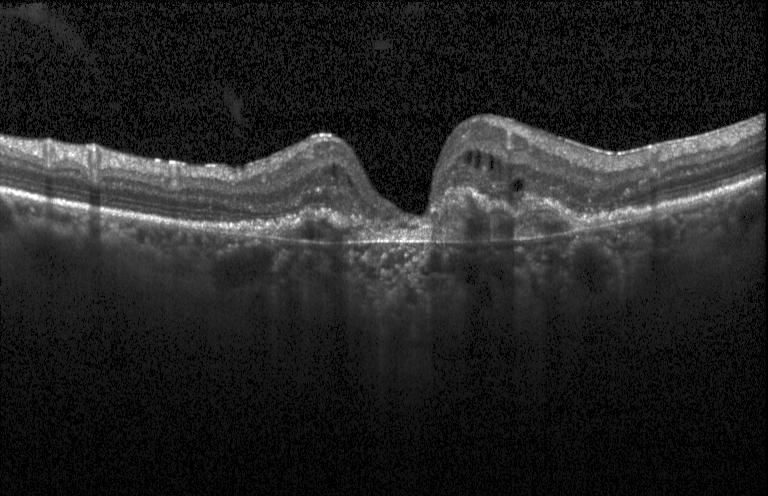
Macular OCT demonstrating a choroidal neovascular membrane.